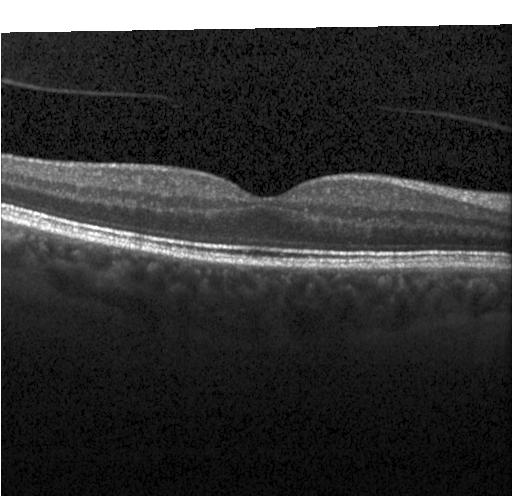

OCT B-scan showing neither choroidal neovascularization, diabetic macular edema, nor drusen.